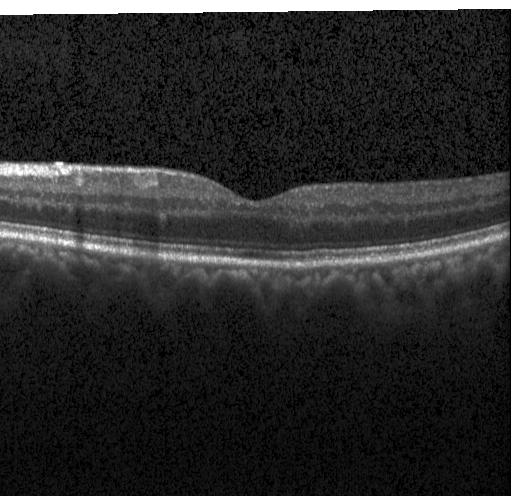 Spectral-domain optical coherence tomography; optical coherence tomography B-scan; fovea-centered; Heidelberg Spectralis. Assessment: neither CNV, DME, nor drusen.